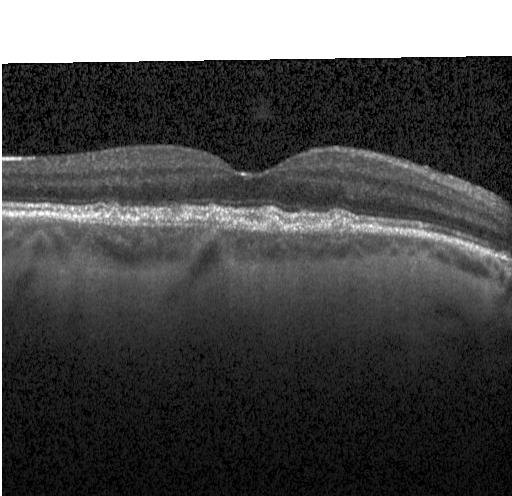

Retinal OCT cross-section showing drusen.